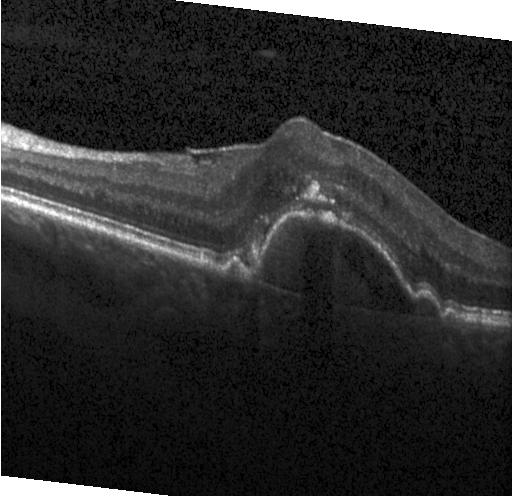 OCT B-scan showing choroidal neovascularization.